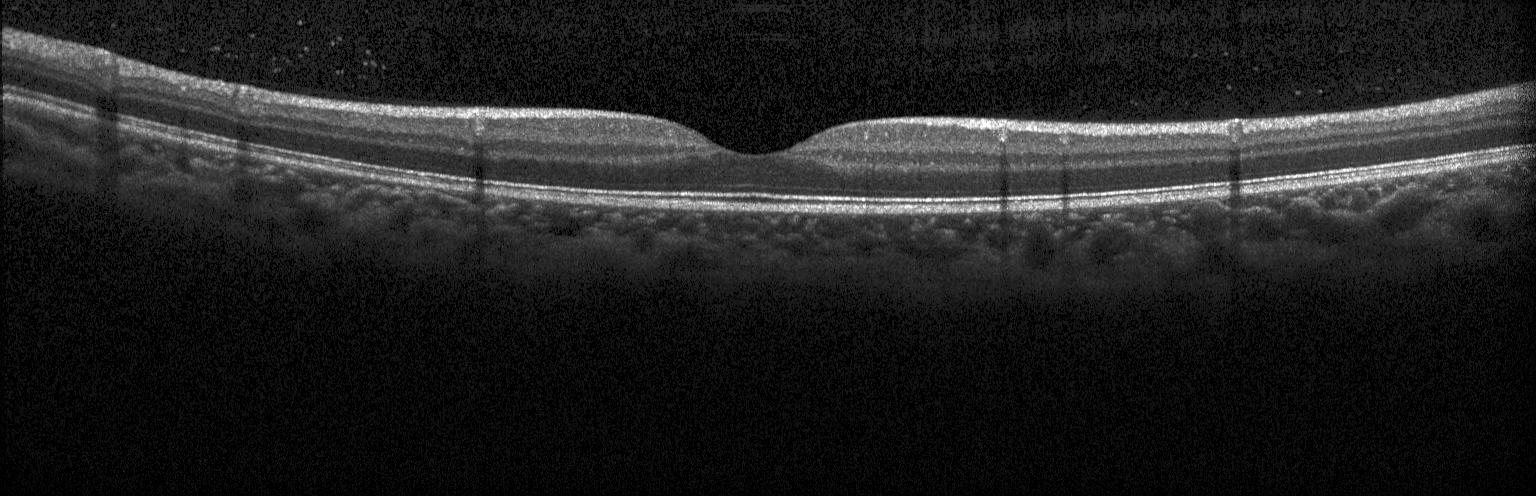
Dx: no choroidal neovascularization, diabetic macular edema, or drusen.